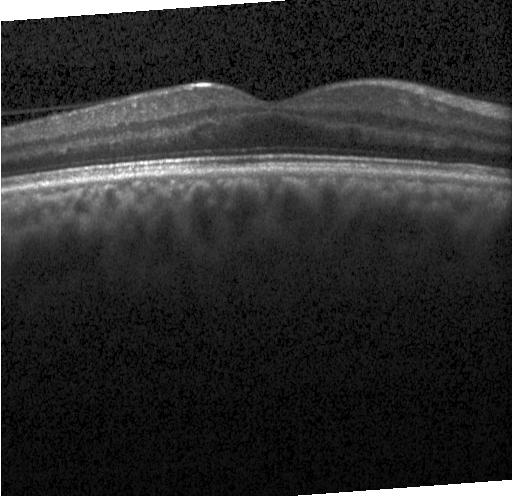 Optical coherence tomography B-scan; centered on the fovea
Macular OCT: no choroidal neovascularization, no diabetic macular edema, and no drusen.